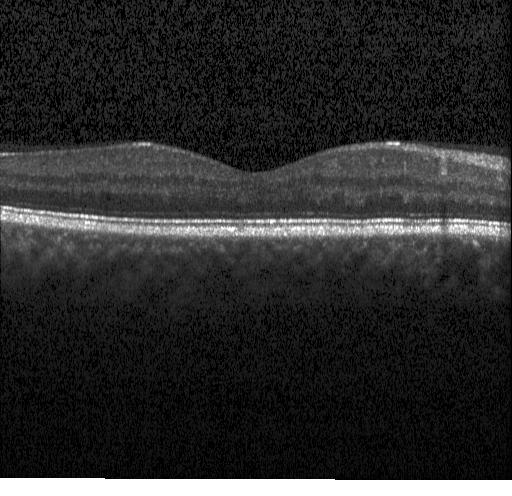

Optical coherence tomography B-scan.
No choroidal neovascularization, diabetic macular edema, or drusen.